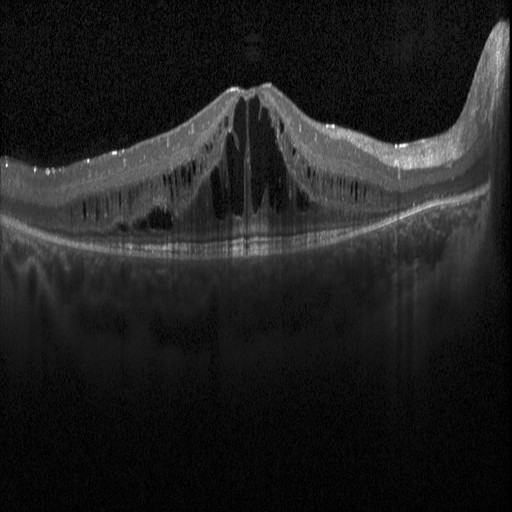 The scan shows DME.